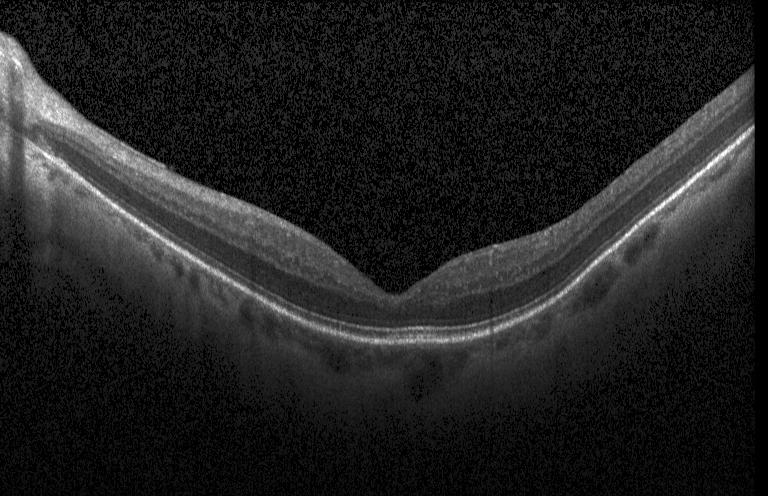

Optical coherence tomography B-scan
Neither choroidal neovascularization, diabetic macular edema, nor drusen.